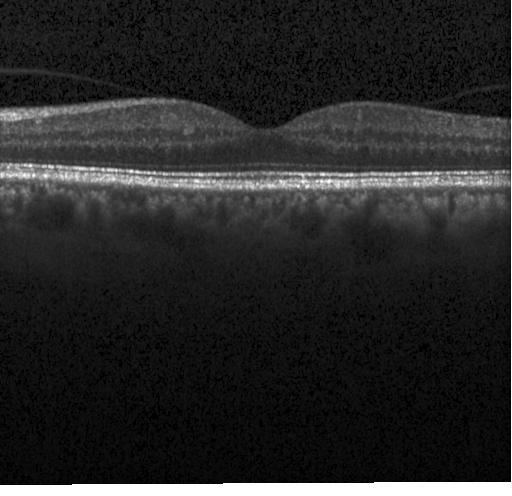

Optical coherence tomography B-scan, instrument: Heidelberg Spectralis, macular scan. Diagnosis: neither choroidal neovascularization, diabetic macular edema, nor drusen.